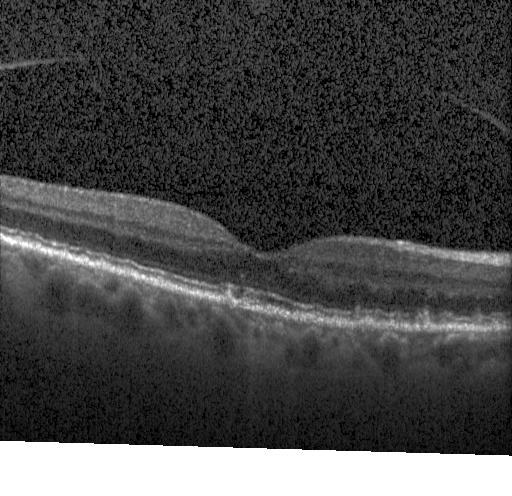
OCT B-scan
The scan shows multiple drusen.